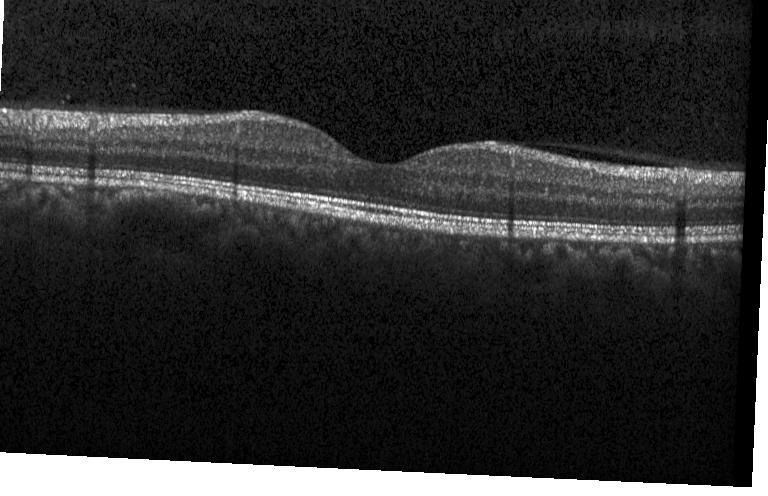

Macular scan, retinal OCT cross-section, Heidelberg Spectralis, spectral-domain OCT. Finding: no evidence of choroidal neovascularization, diabetic macular edema, or drusen.